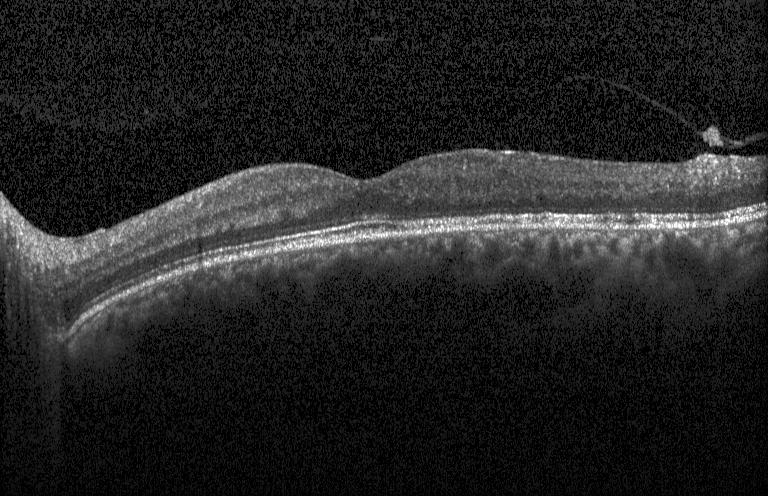

Dx: neither CNV, DME, nor drusen.